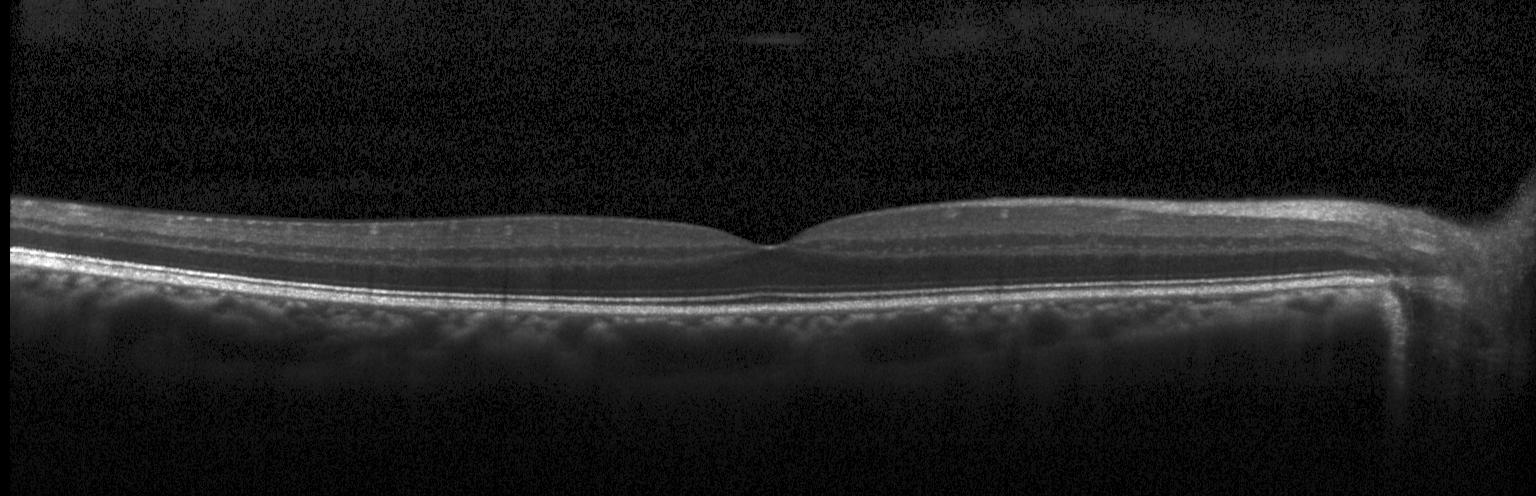 This B-scan demonstrates neither CNV, DME, nor drusen.